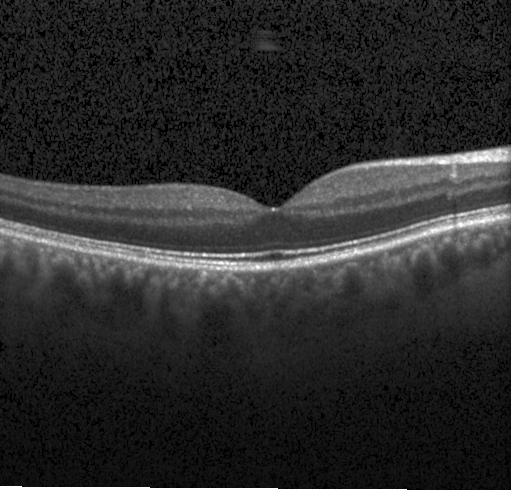 OCT line scan, acquired on a Heidelberg Spectralis — This B-scan demonstrates no CNV, DME, or drusen.